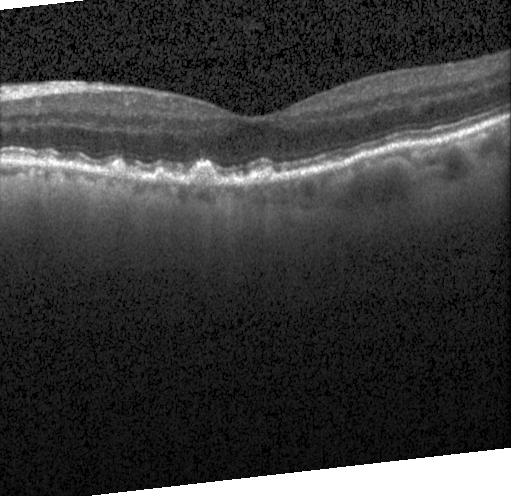

Optical coherence tomography scan
The scan shows drusen.